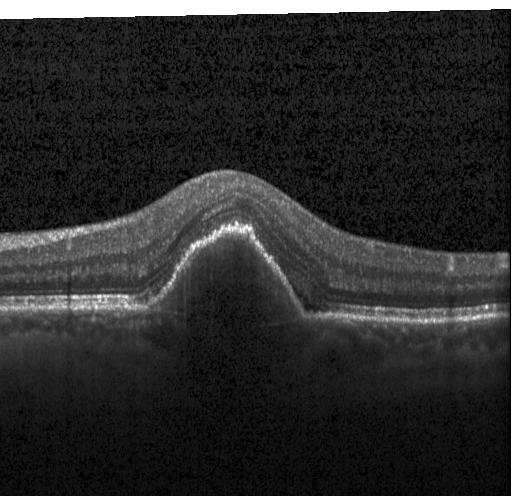

Centered on the fovea. Acquired on a Heidelberg Spectralis. Optical coherence tomography B-scan — Diagnosis: choroidal neovascularization.